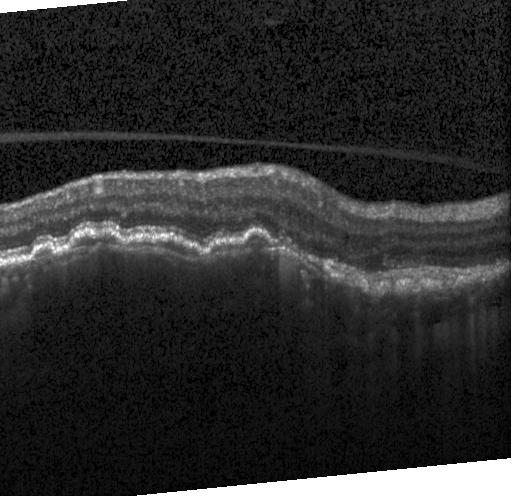
Impression: CNV.